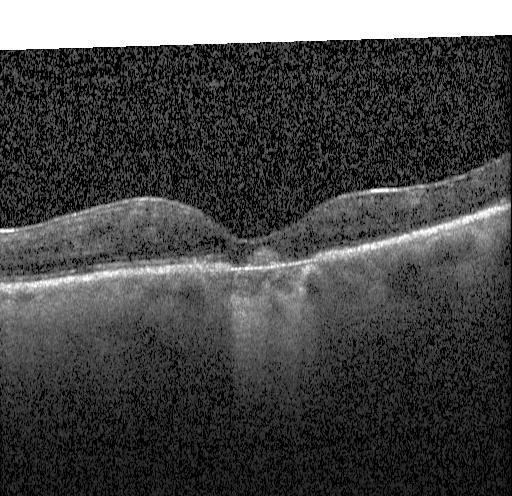

Dx: a choroidal neovascular membrane.